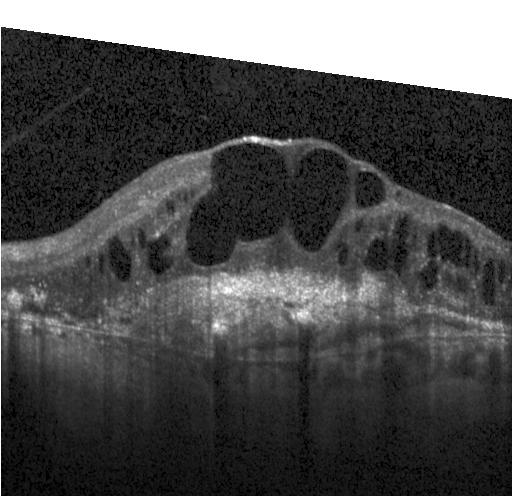 Heidelberg Spectralis; optical coherence tomography scan; SD-OCT; fovea-centered
Finding: a choroidal neovascular membrane.